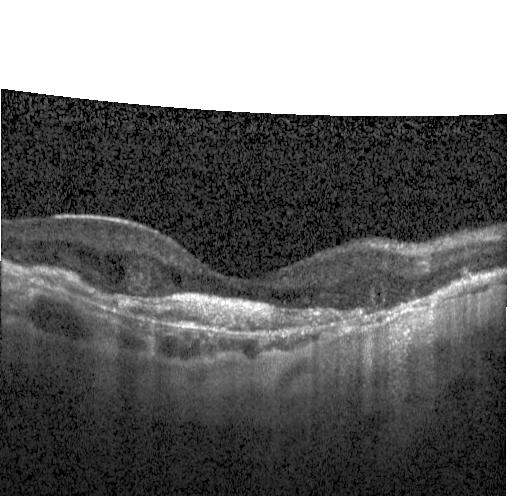
Impression: a choroidal neovascular membrane.